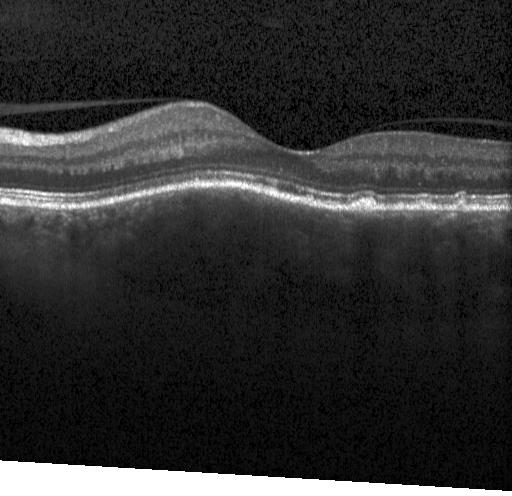
This B-scan demonstrates multiple drusen.